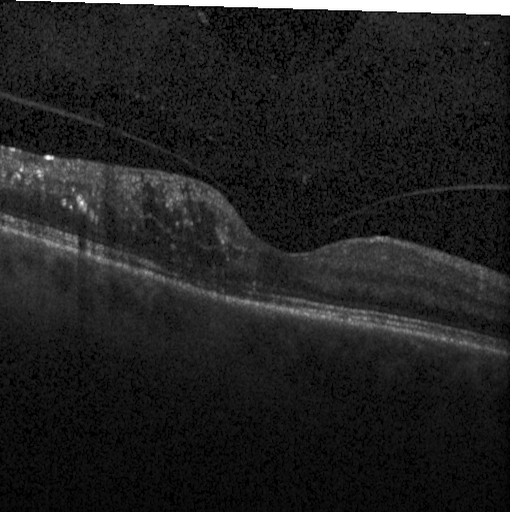

The scan shows diabetic macular edema (DME).